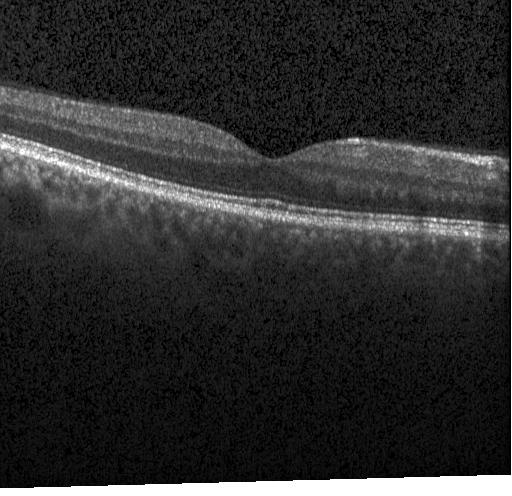
Impression: no evidence of CNV, DME, or drusen.